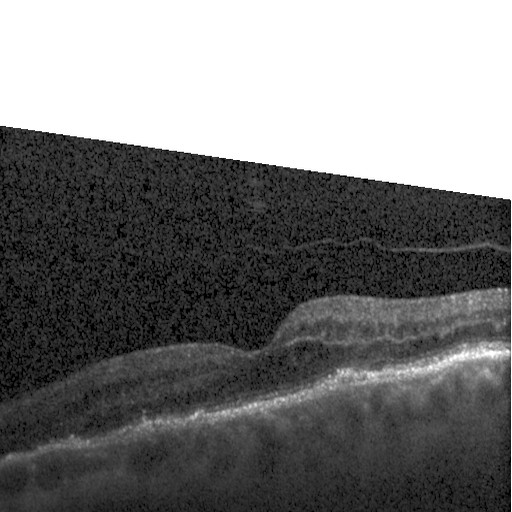

Diagnosis: DME.